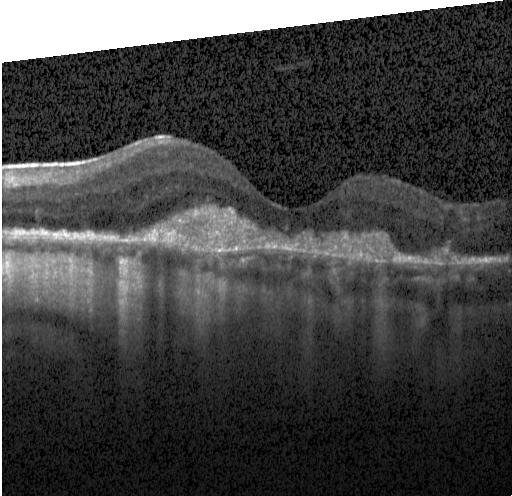

Optical coherence tomography B-scan. Impression: CNV.